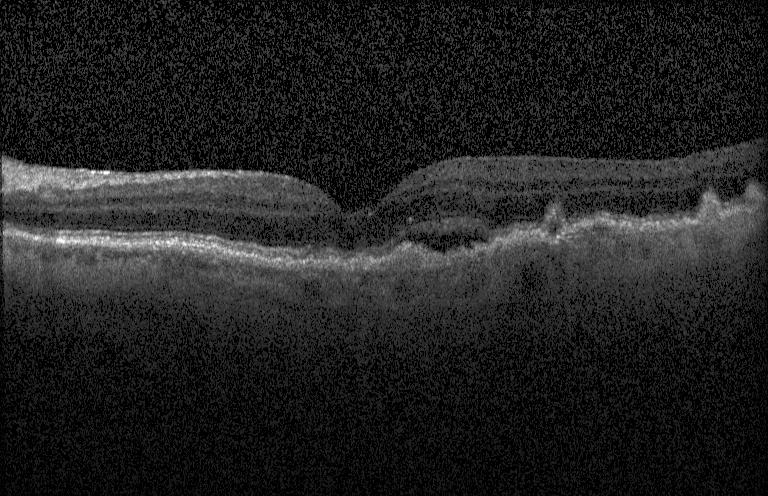

SD-OCT, OCT line scan, fovea-centered, Heidelberg Spectralis OCT system — OCT finding: CNV.